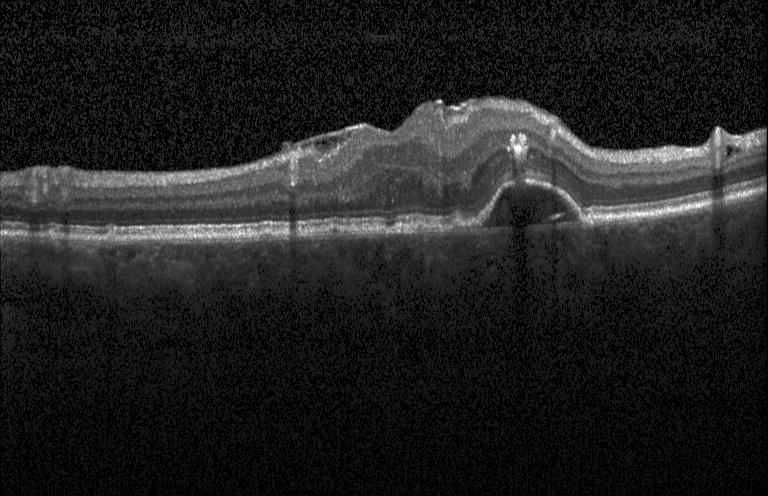 Macular OCT: a choroidal neovascular membrane.